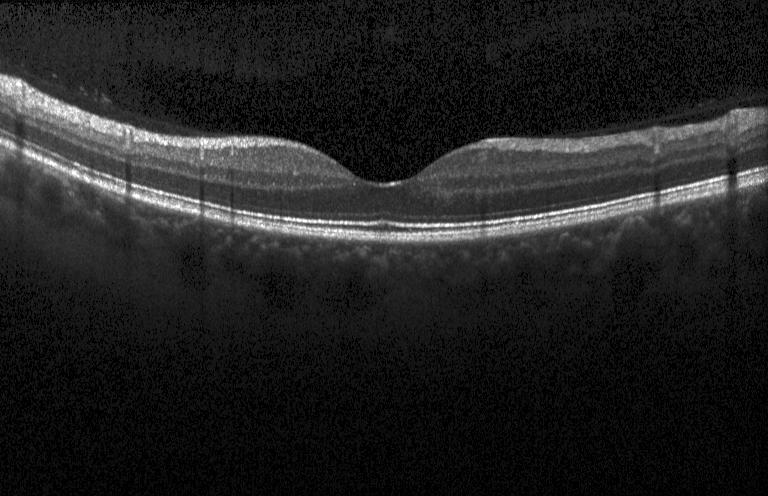

Optical coherence tomography scan. Impression: no evidence of CNV, DME, or drusen.